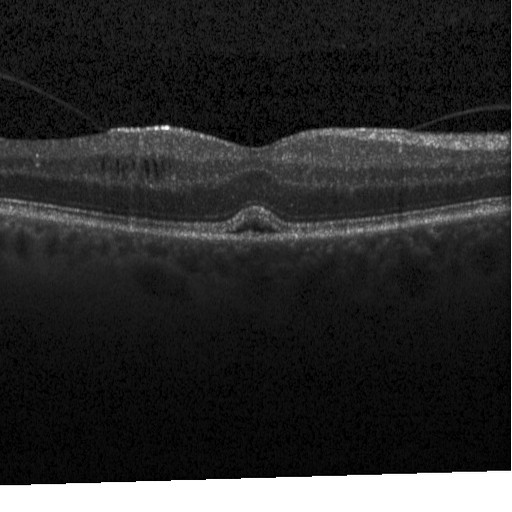
Optical coherence tomography B-scan; centered on the fovea; Heidelberg Spectralis; SD-OCT — Diagnosis: DME.